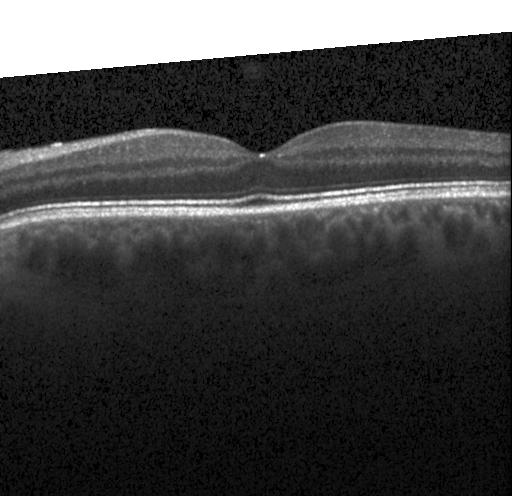

Acquired on a Heidelberg Spectralis; OCT B-scan
No choroidal neovascularization, diabetic macular edema, or drusen.